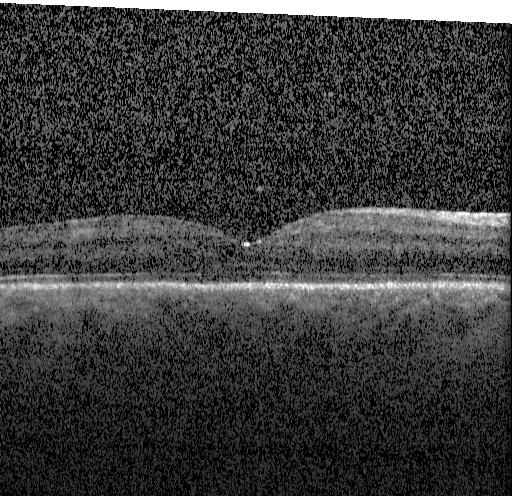

Optical coherence tomography scan. Impression: no choroidal neovascularization, no diabetic macular edema, and no drusen.